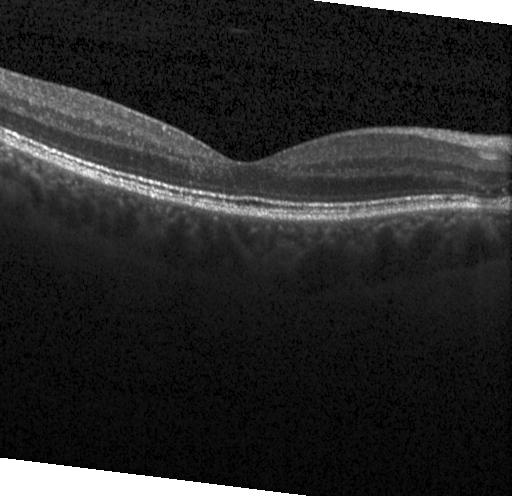
OCT line scan.
Diagnosis: no choroidal neovascularization, diabetic macular edema, or drusen.